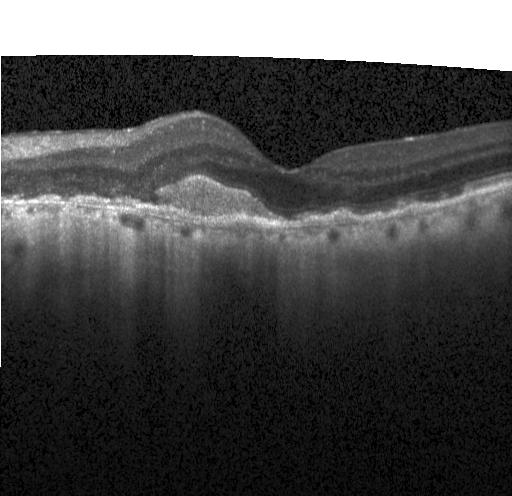
Retinal OCT B-scan — This B-scan demonstrates choroidal neovascularization (CNV).